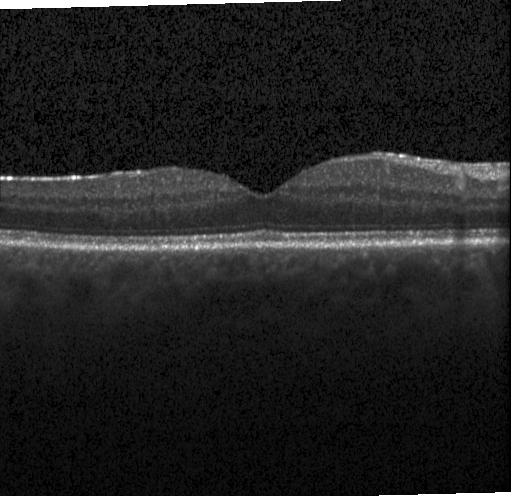

Assessment: no choroidal neovascularization, no diabetic macular edema, and no drusen.